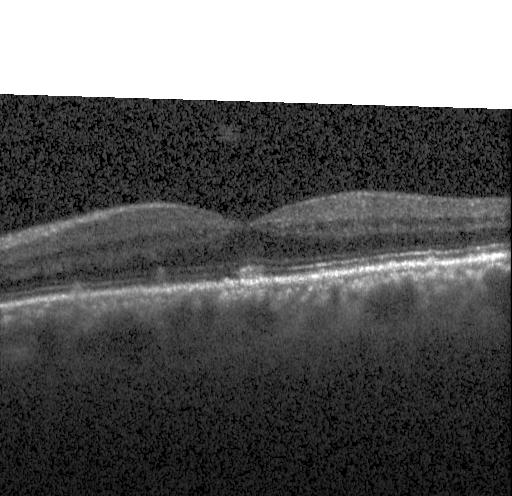 Macular scan · spectral-domain OCT · Heidelberg Spectralis OCT system · optical coherence tomography scan. OCT finding: drusen.